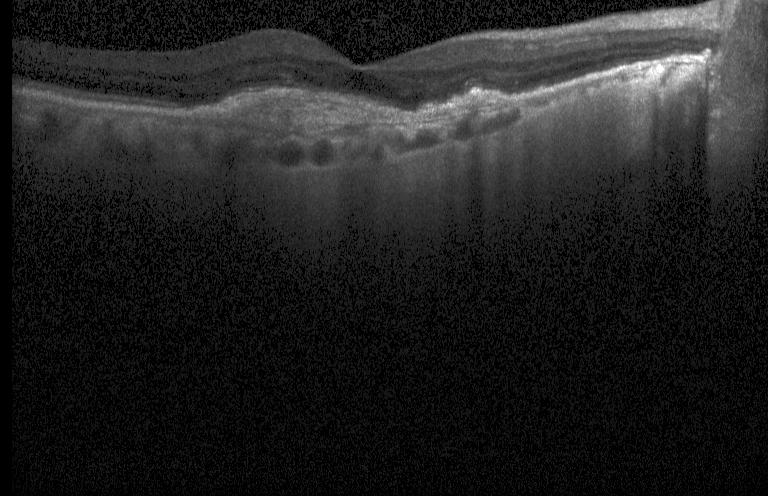

Optical coherence tomography scan
Dx: choroidal neovascularization (CNV).